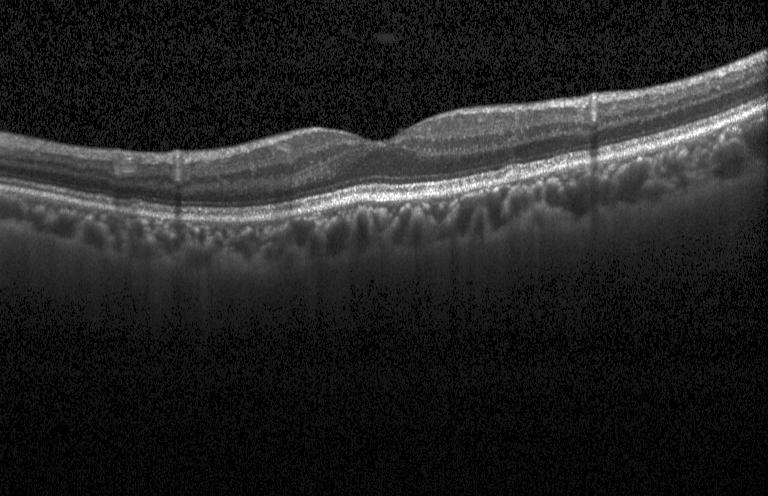

Impression: no evidence of CNV, DME, or drusen.